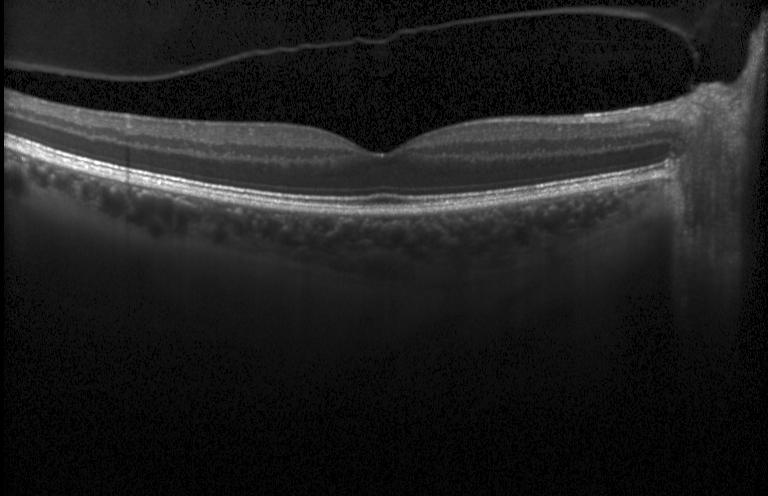 Optical coherence tomography scan, Heidelberg Spectralis.
Impression: no choroidal neovascularization, no diabetic macular edema, and no drusen.